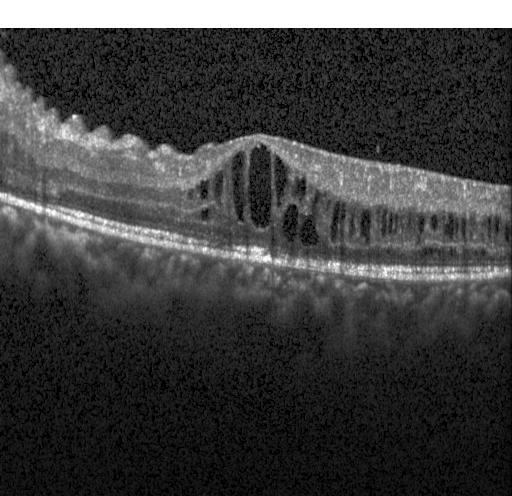
Diagnosis: diabetic macular edema.